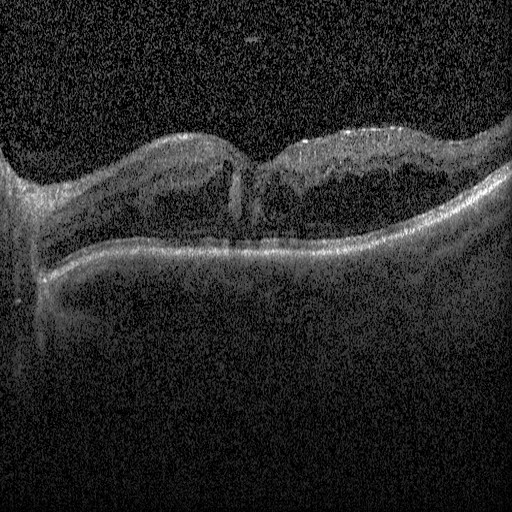

Retinal OCT B-scan. OCT finding: diabetic macular edema.